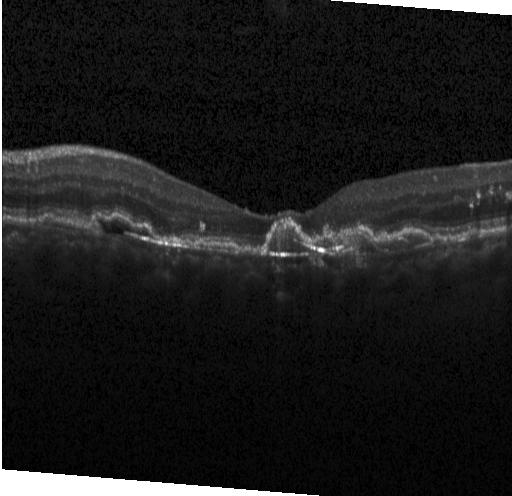

Diagnosis: choroidal neovascularization (CNV).